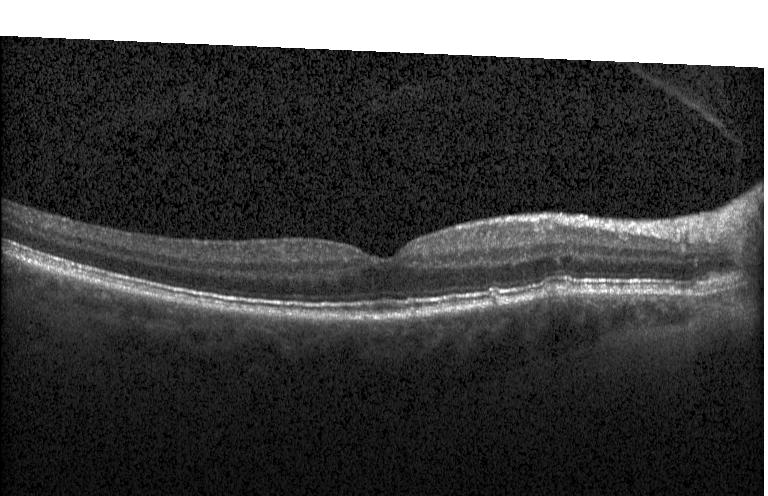 Retinal OCT cross-section. Diagnosis: drusen.